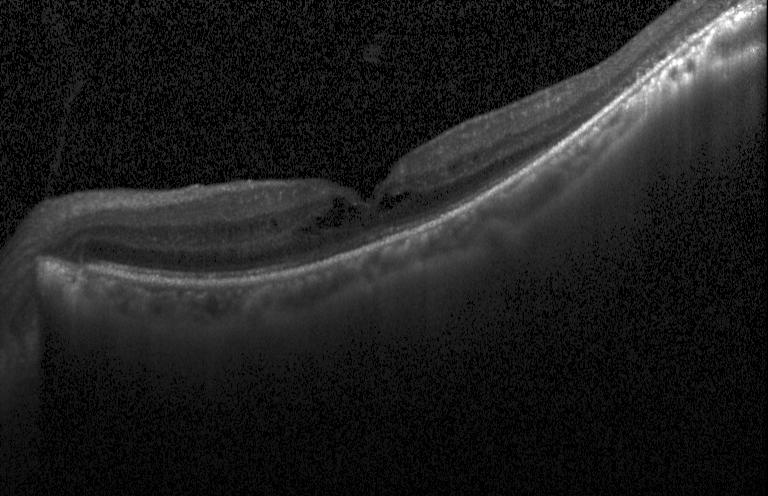

Spectral-domain OCT; OCT B-scan. Impression: diabetic macular edema (DME).